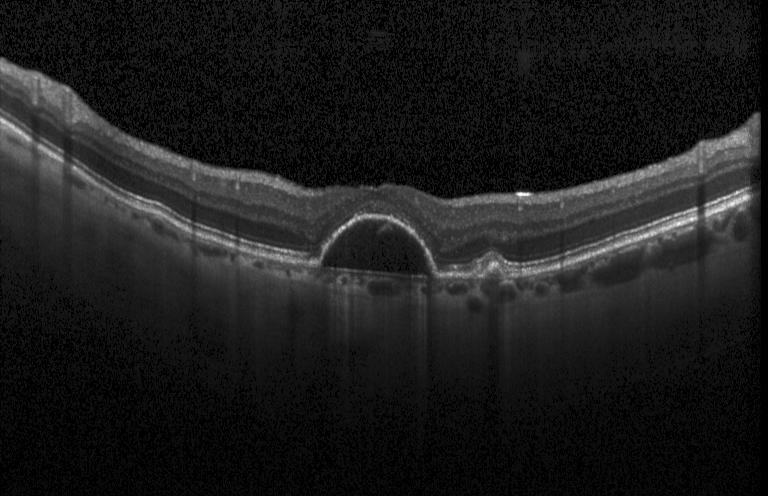

Dx: choroidal neovascularization (CNV).